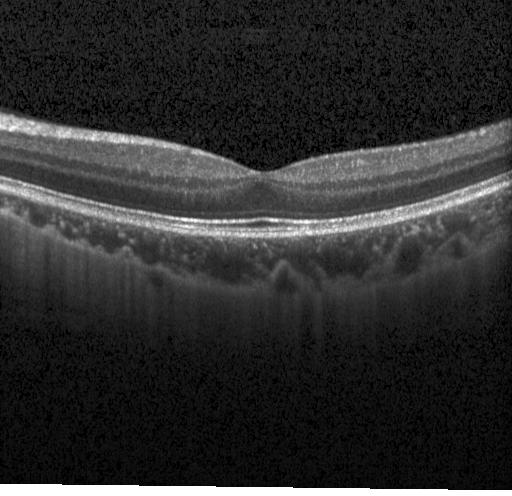
Fovea-centered; OCT line scan
The scan shows no CNV, no DME, and no drusen.